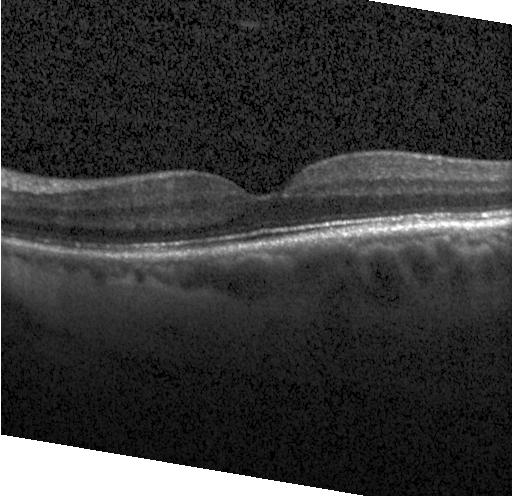 Fovea-centered. OCT line scan.
OCT finding: no CNV, no DME, and no drusen.